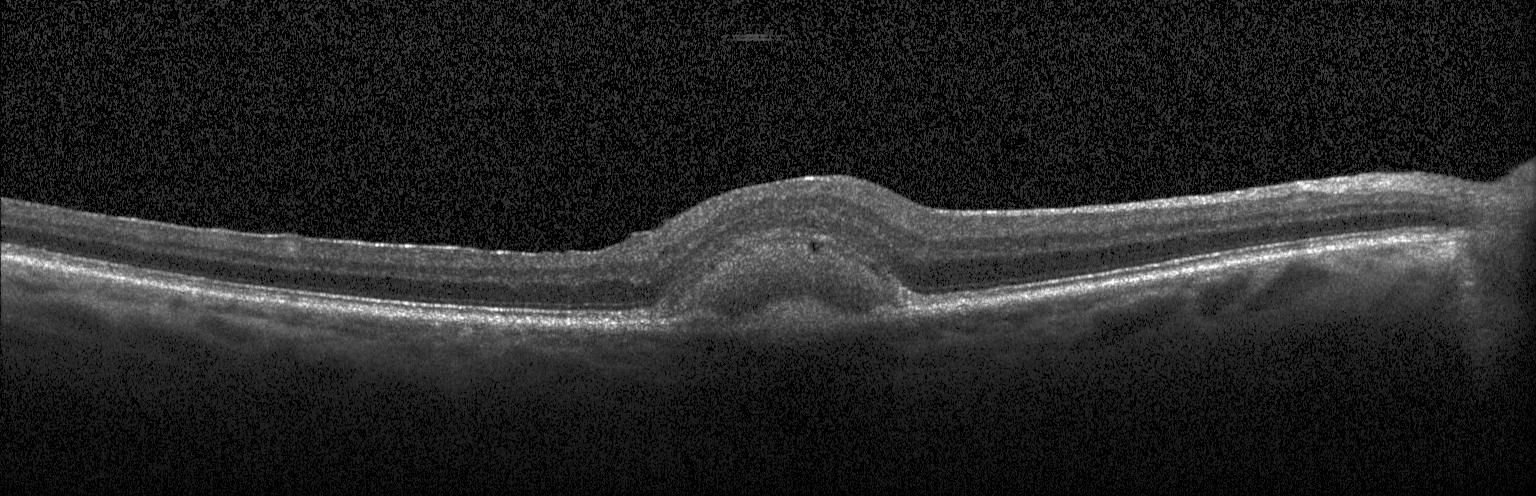 Macular OCT: choroidal neovascularization.